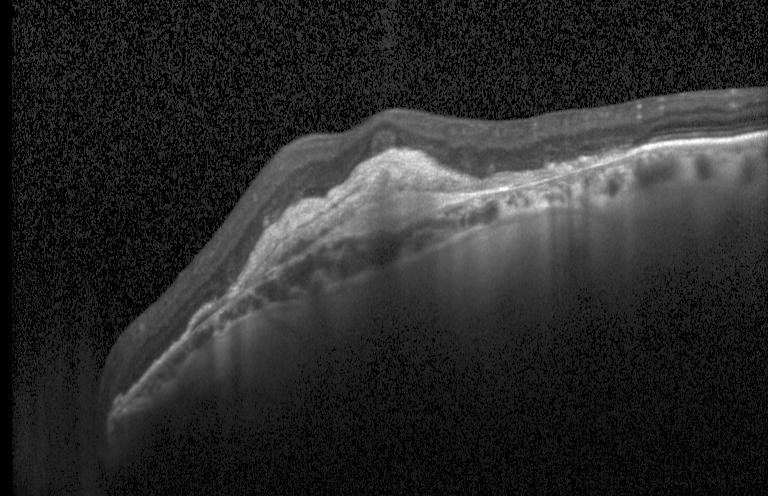
Assessment: choroidal neovascularization (CNV).